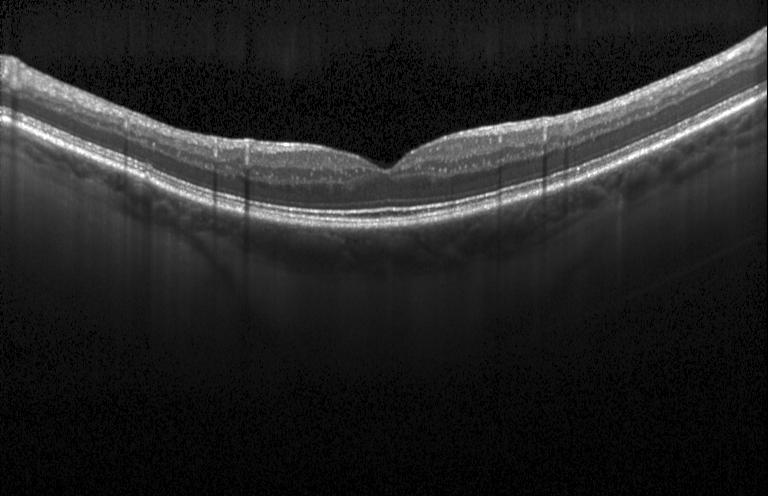 Spectral-domain OCT, through the macula, Heidelberg Spectralis, optical coherence tomography scan — The scan shows neither CNV, DME, nor drusen.